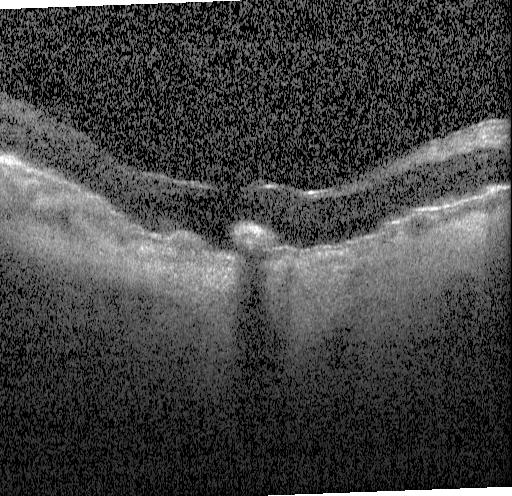
Retinal OCT cross-section; Heidelberg Spectralis OCT system; spectral-domain optical coherence tomography
This B-scan demonstrates CNV.